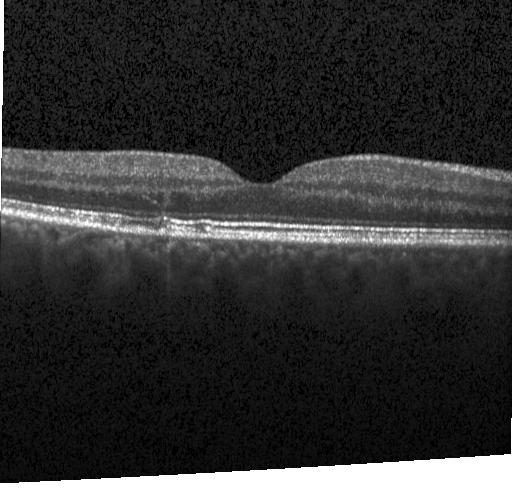

Impression: no evidence of choroidal neovascularization, diabetic macular edema, or drusen.